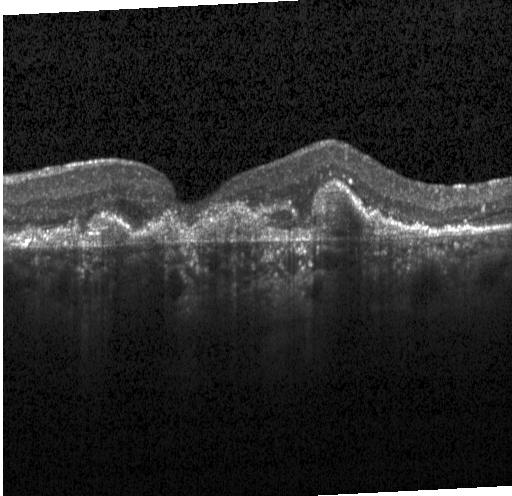 Retinal OCT B-scan.
Impression: choroidal neovascularization.